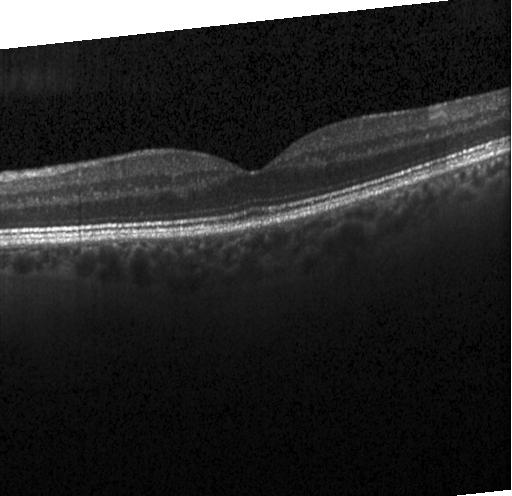
No choroidal neovascularization, diabetic macular edema, or drusen.